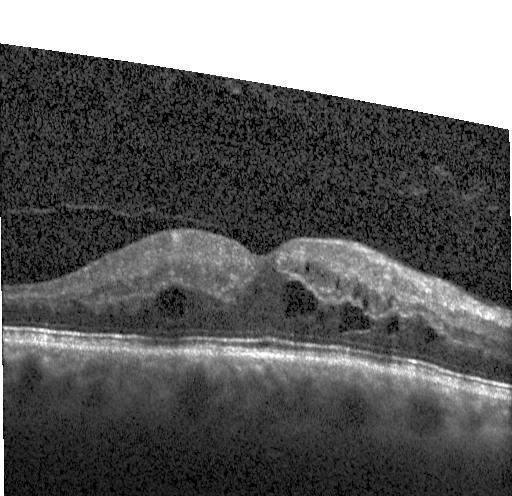
Macular OCT: DME.